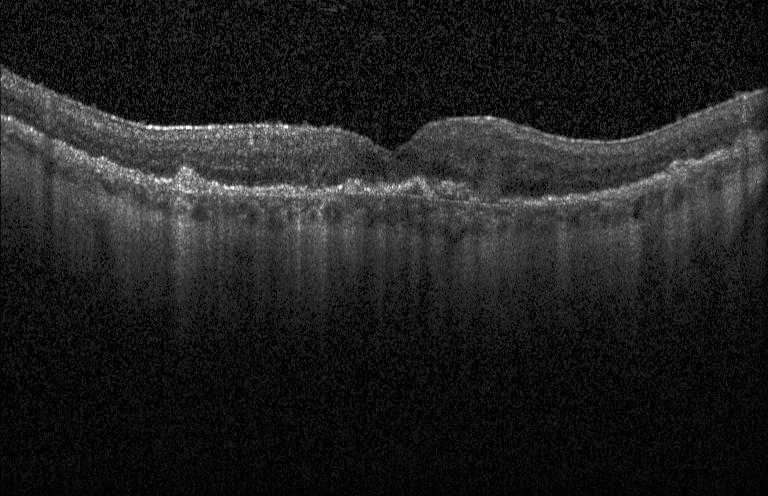

Through the macula · OCT B-scan · Heidelberg Spectralis · spectral-domain OCT — Dx: CNV.